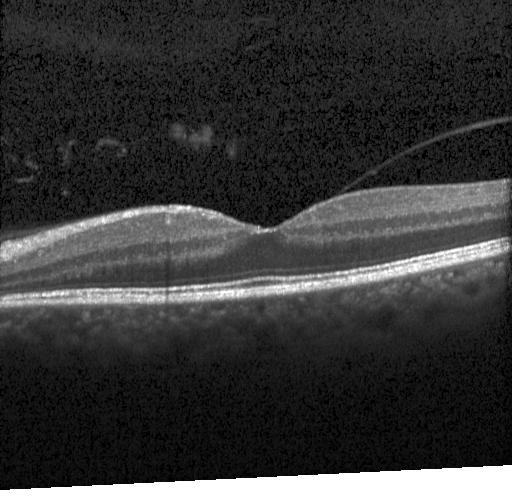

Through the macula; retinal OCT B-scan
The scan shows neither choroidal neovascularization, diabetic macular edema, nor drusen.